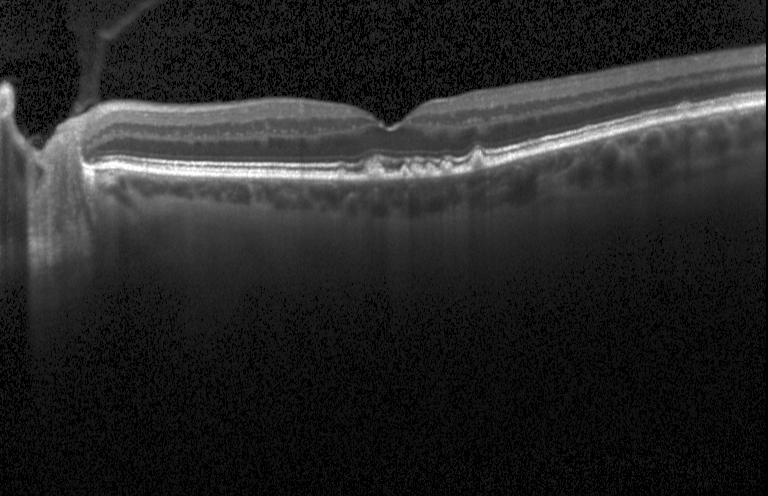
Assessment: multiple drusen.